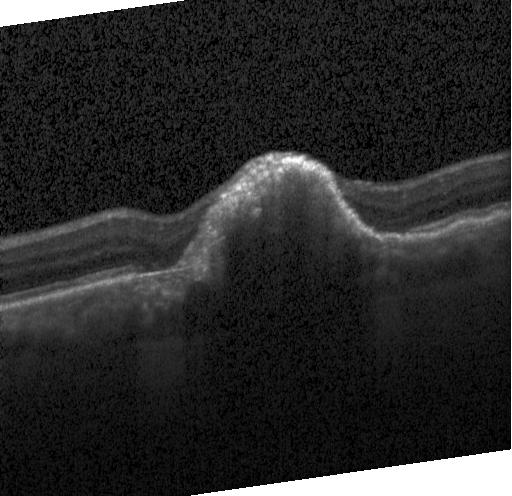 Finding: CNV.